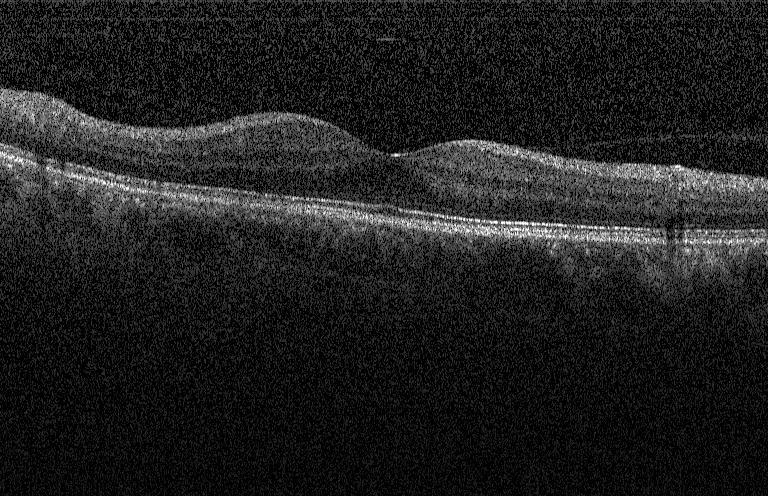

Heidelberg Spectralis OCT system · OCT B-scan
OCT finding: neither CNV, DME, nor drusen.